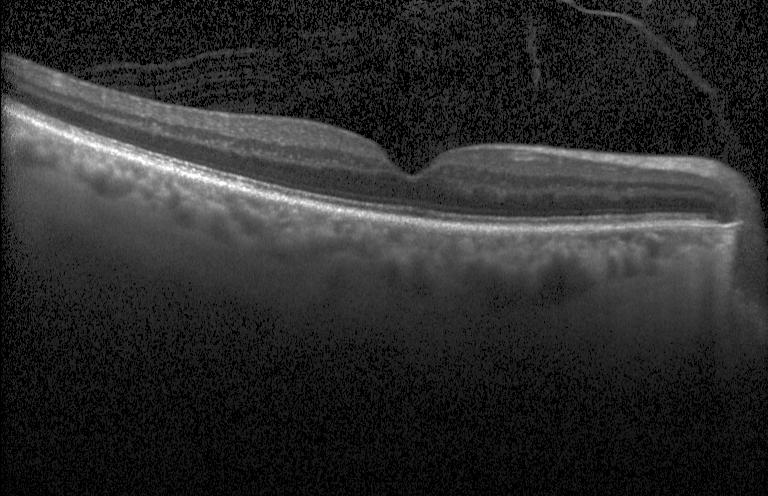 Dx: no CNV, DME, or drusen.